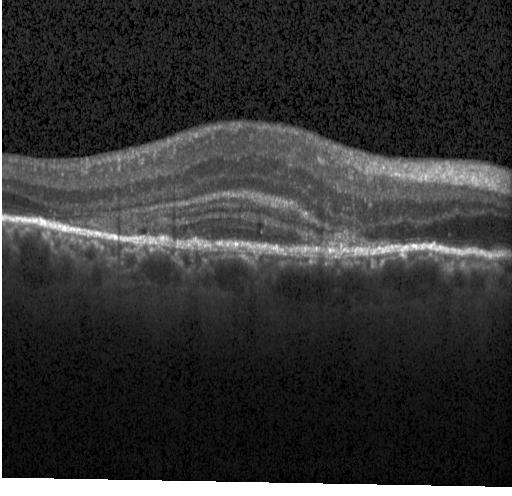

Optical coherence tomography scan
Impression: choroidal neovascularization.